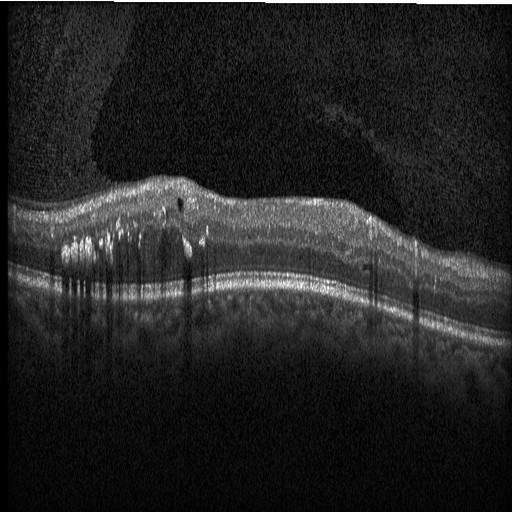

OCT B-scan. Heidelberg Spectralis. SD-OCT
Macular OCT: DME.